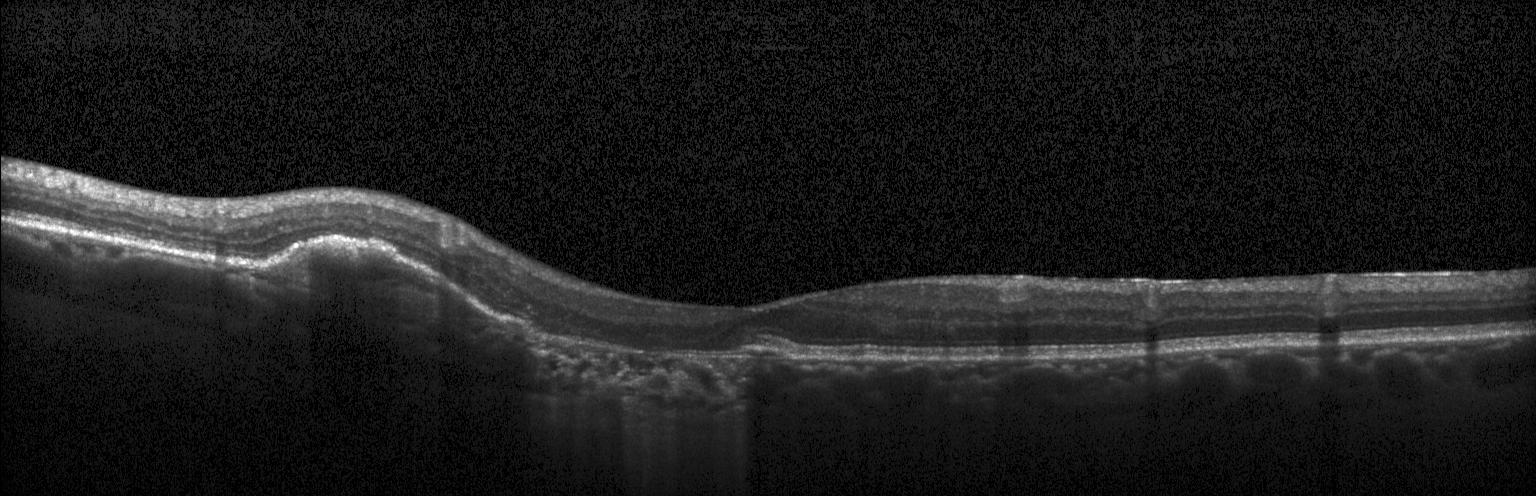 Centered on the fovea; OCT line scan; spectral-domain optical coherence tomography; Heidelberg Spectralis — Macular OCT: a choroidal neovascular membrane.